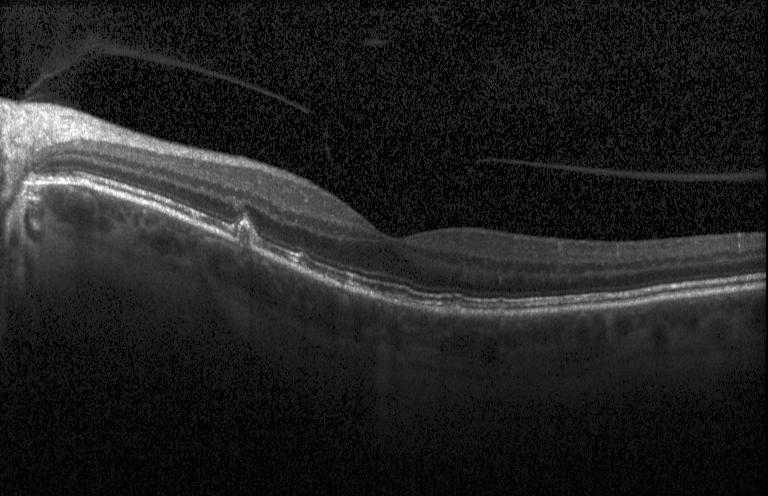
Spectral-domain optical coherence tomography, Heidelberg Spectralis, retinal OCT B-scan, macular scan.
Drusen.